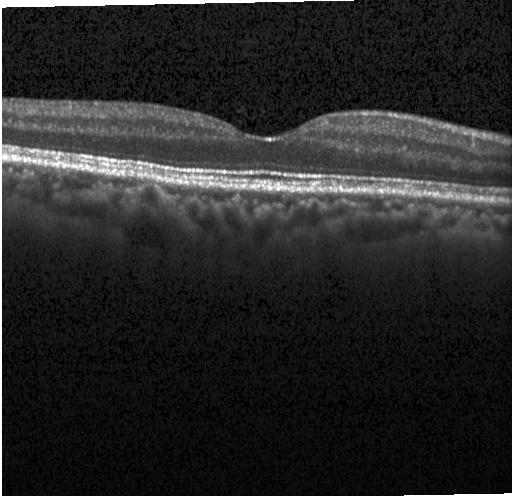 Impression: no evidence of choroidal neovascularization, diabetic macular edema, or drusen.